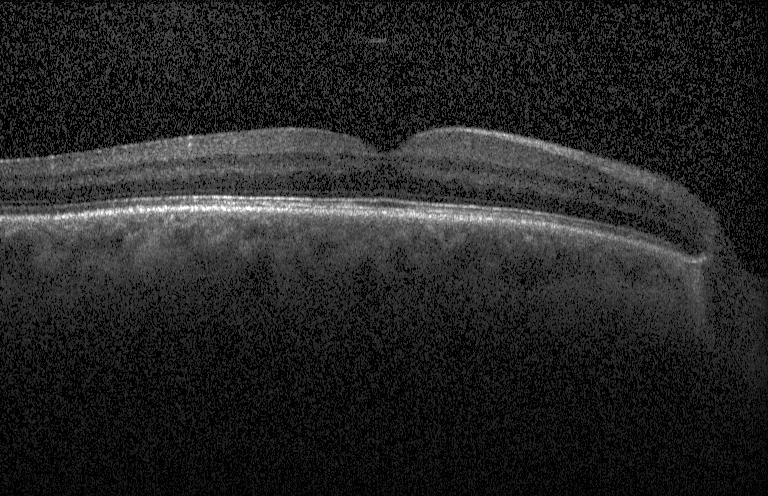 Retinal OCT cross-section showing neither CNV, DME, nor drusen.